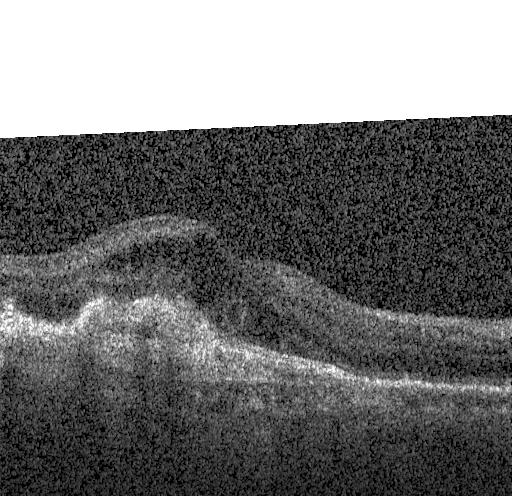 This B-scan demonstrates choroidal neovascularization.